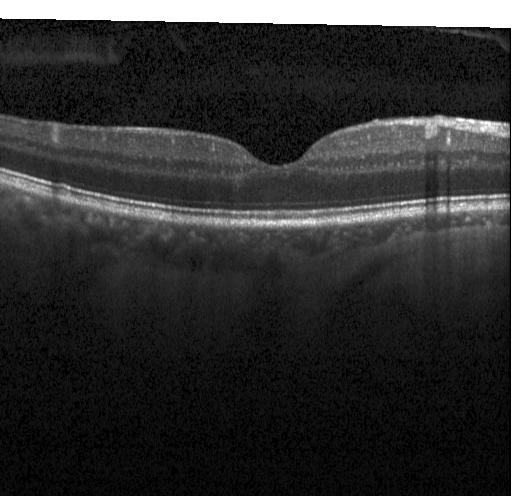
Optical coherence tomography B-scan.
This B-scan demonstrates no choroidal neovascularization, diabetic macular edema, or drusen.